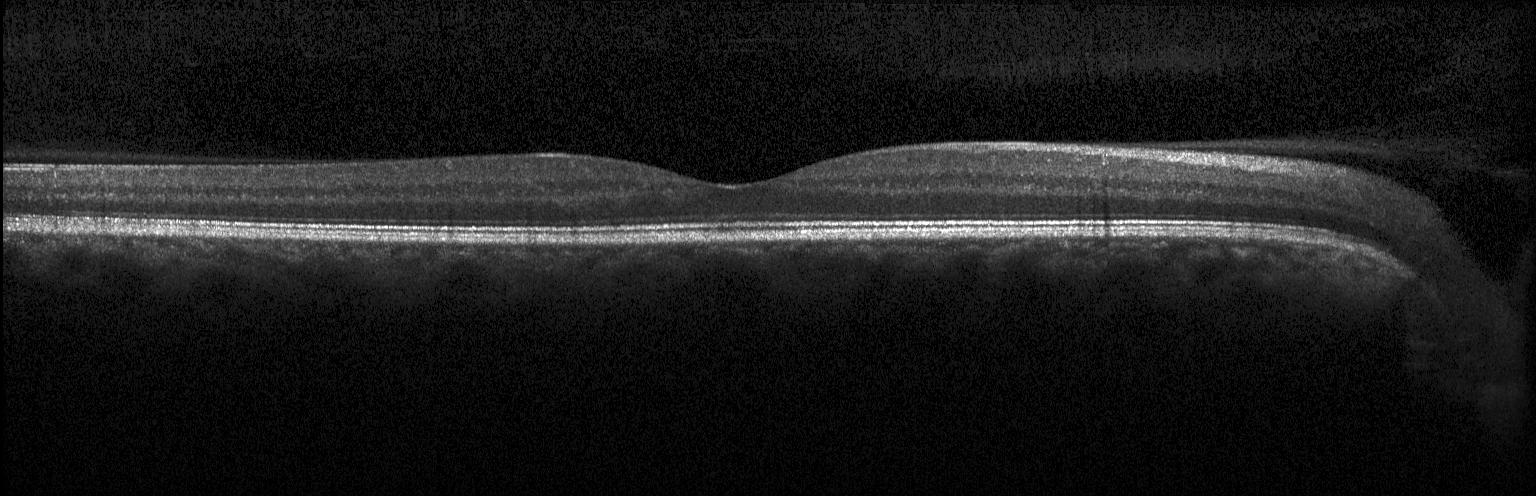
Optical coherence tomography B-scan. Finding: no choroidal neovascularization, diabetic macular edema, or drusen.